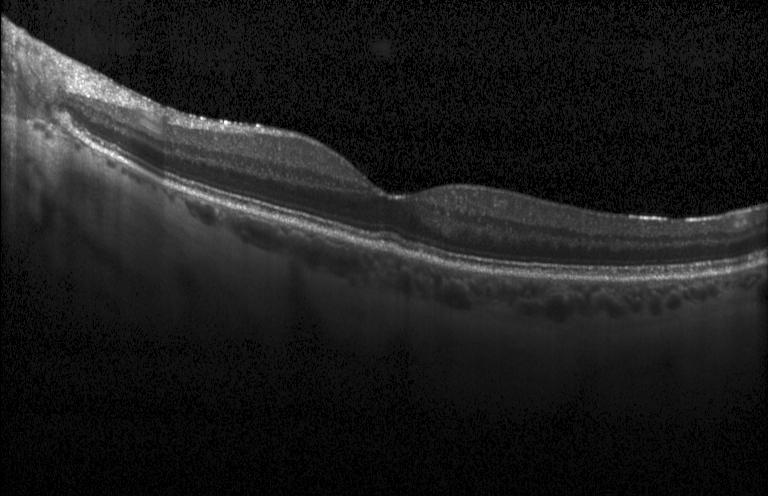 SD-OCT; optical coherence tomography scan.
Finding: no choroidal neovascularization, diabetic macular edema, or drusen.